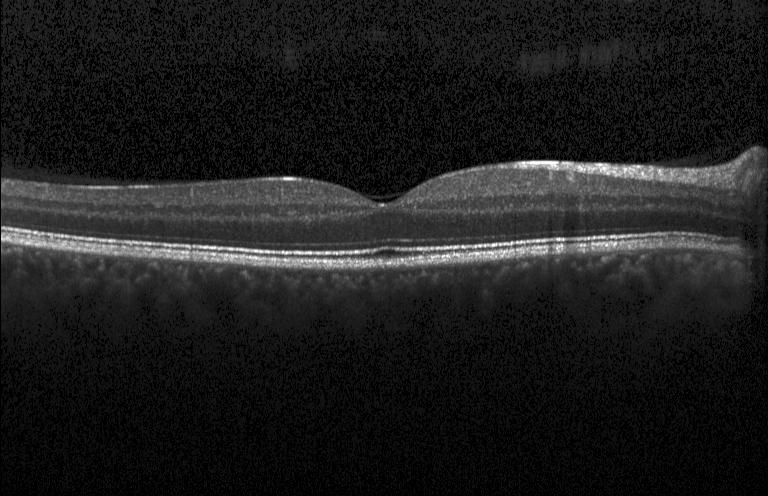
Dx: no choroidal neovascularization, no diabetic macular edema, and no drusen.